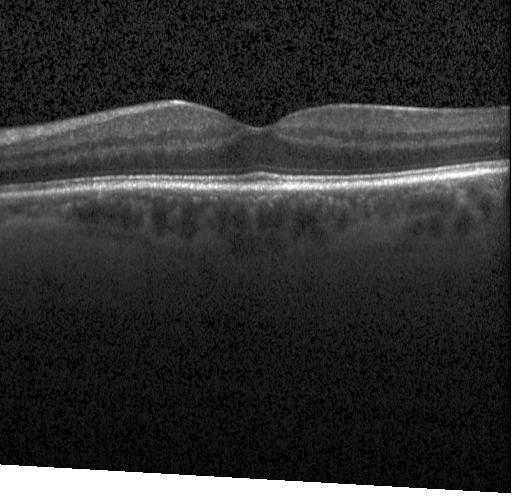 Instrument: Heidelberg Spectralis · spectral-domain OCT · through the macula · optical coherence tomography B-scan
Finding: no evidence of CNV, DME, or drusen.